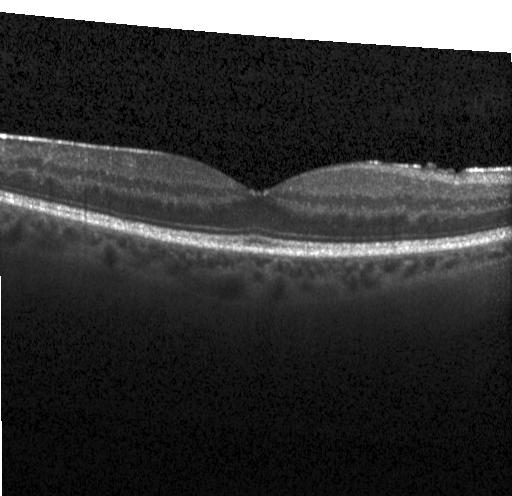

OCT finding: no evidence of CNV, DME, or drusen.